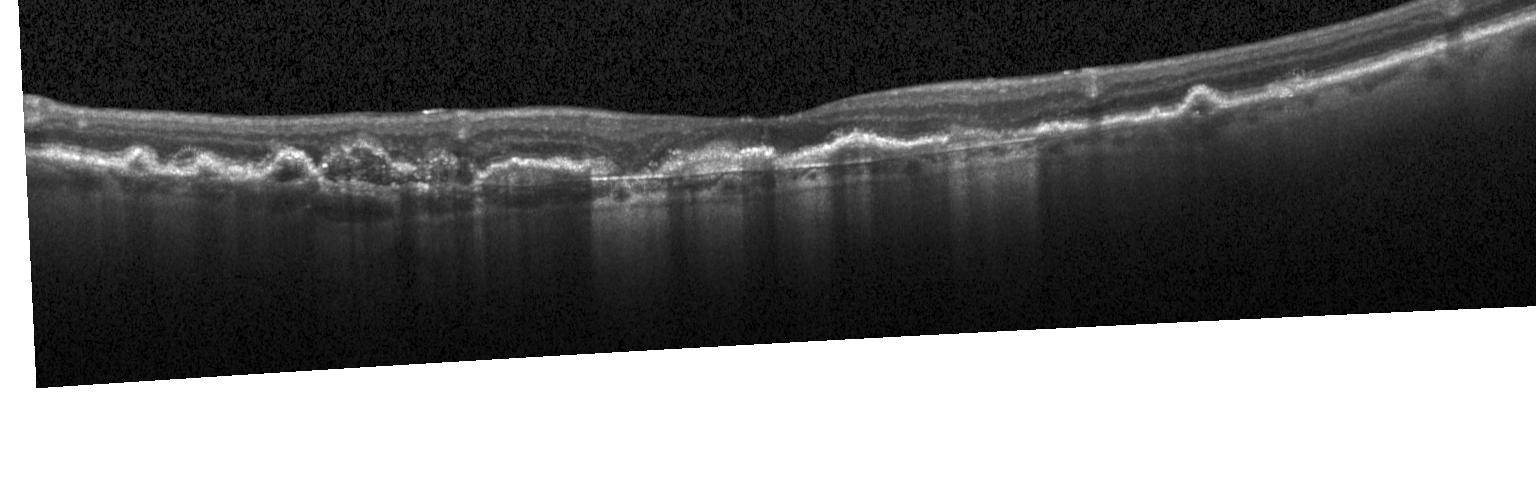
Through the macula, OCT B-scan, instrument: Heidelberg Spectralis. CNV.